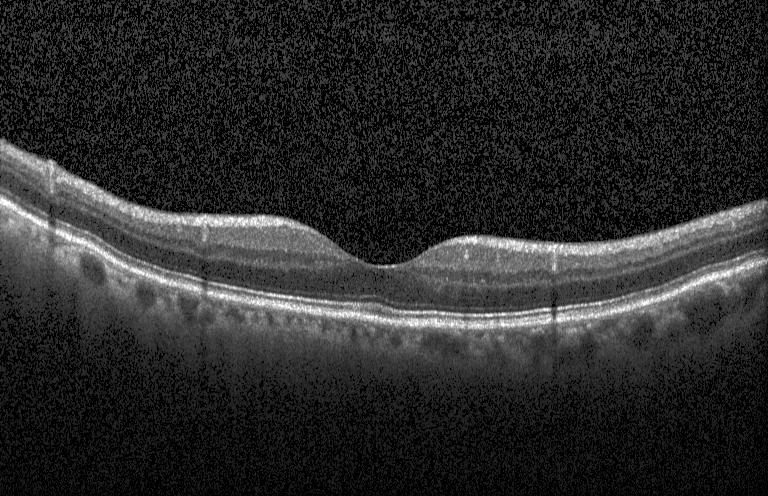

Spectral-domain OCT · retinal OCT cross-section. Impression: no choroidal neovascularization, no diabetic macular edema, and no drusen.